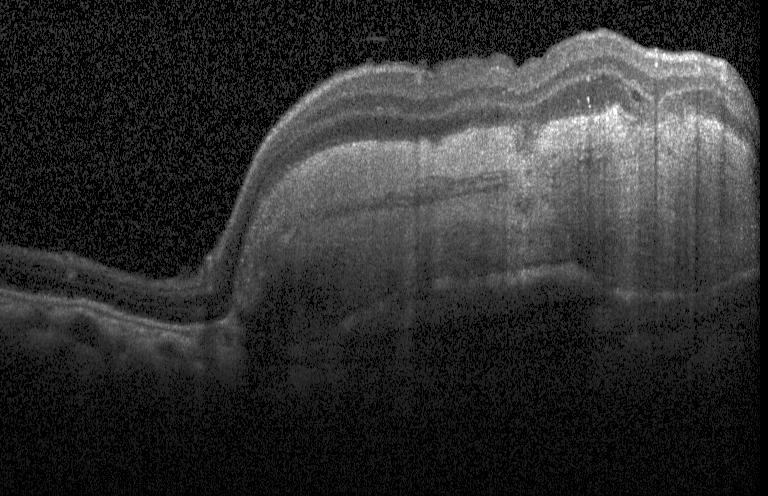

Retinal OCT cross-section
Dx: a choroidal neovascular membrane.